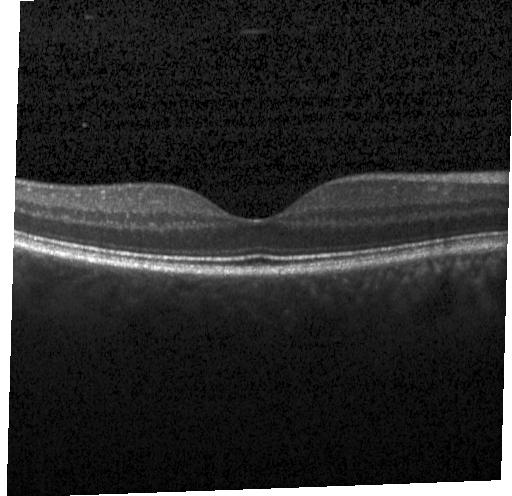 Finding: no CNV, no DME, and no drusen.